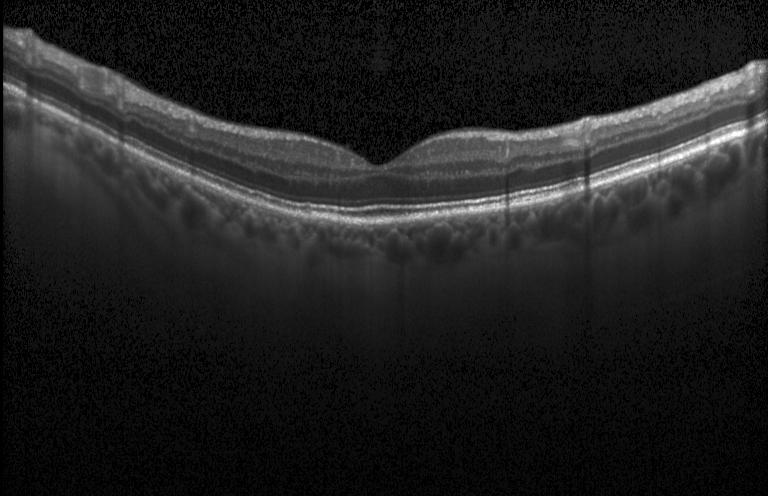 Finding: no choroidal neovascularization, diabetic macular edema, or drusen.